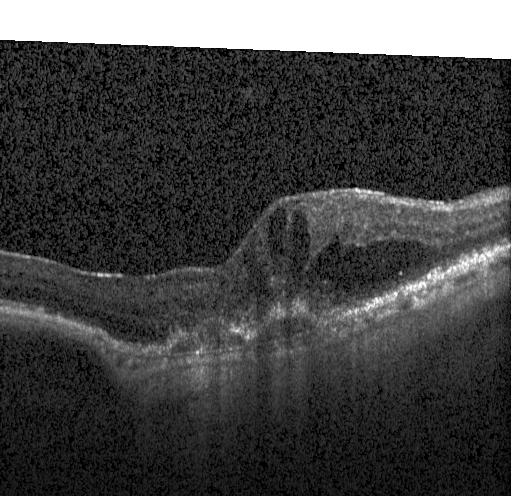
Macular OCT demonstrating a choroidal neovascular membrane.